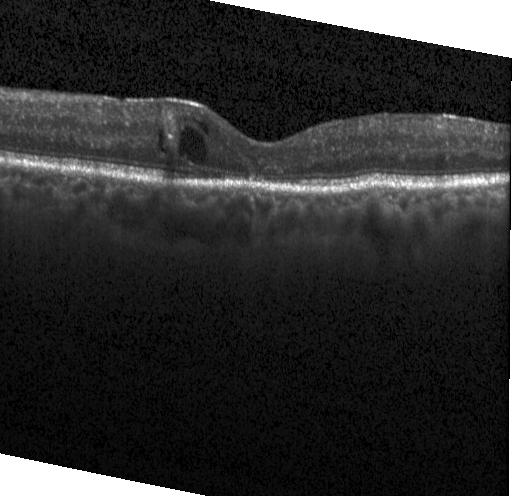
Retinal OCT B-scan. Diabetic macular edema.